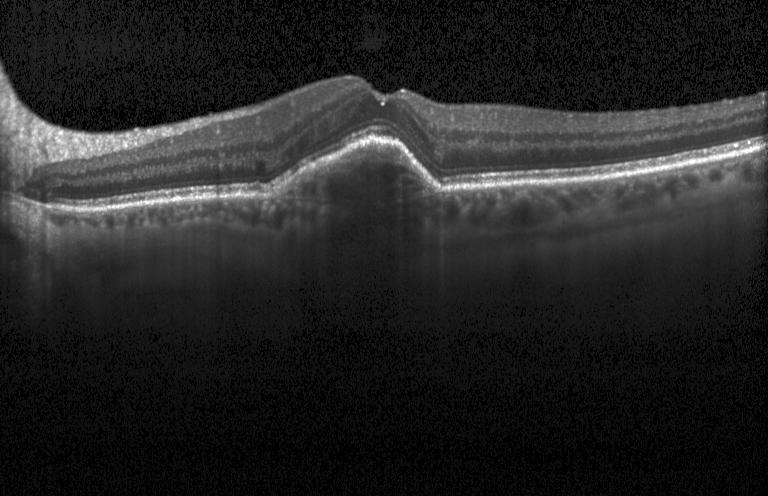
Diagnosis: a choroidal neovascular membrane.